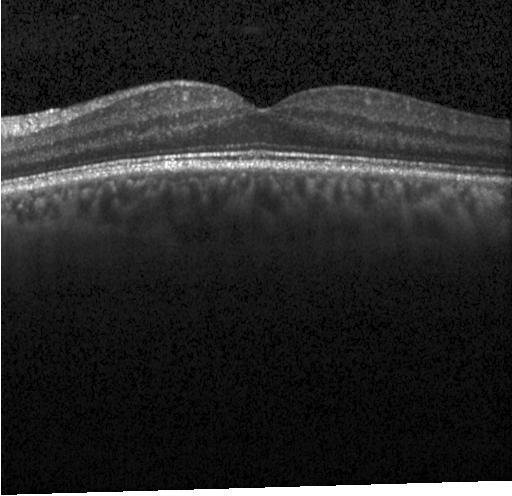 This B-scan demonstrates neither choroidal neovascularization, diabetic macular edema, nor drusen.